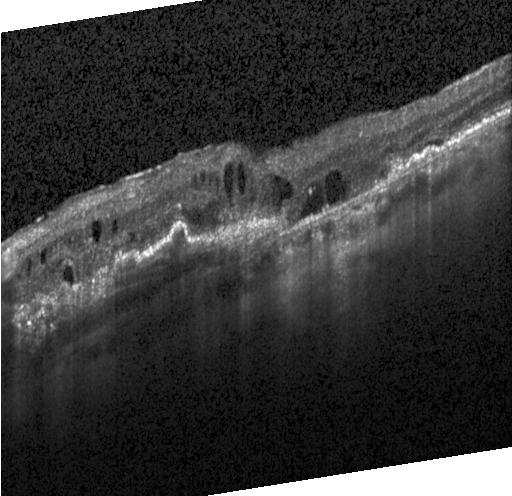 OCT finding: CNV.